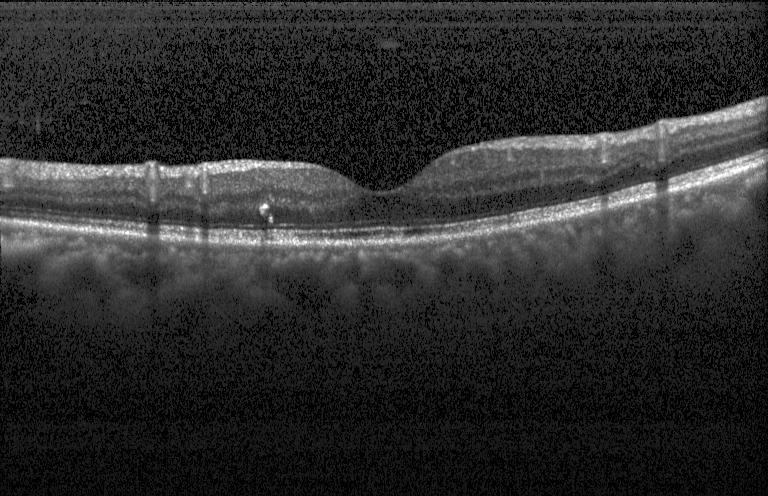
The scan shows diabetic macular edema (DME).